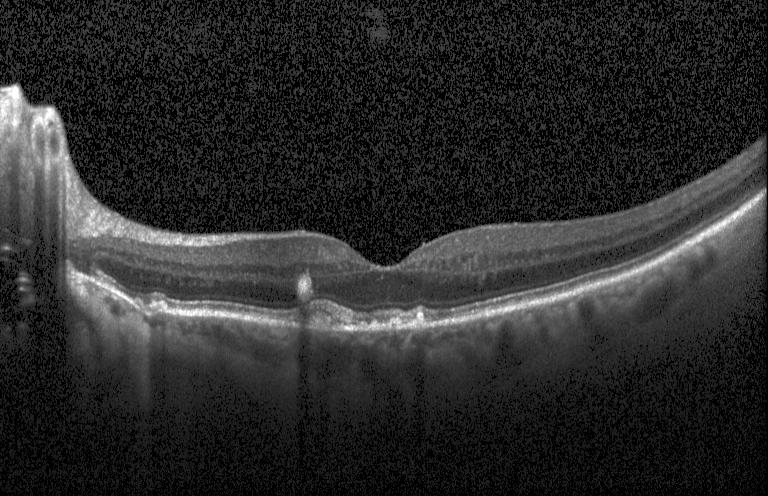 Spectral-domain OCT · retinal OCT B-scan · through the macula
Diagnosis: multiple drusen.